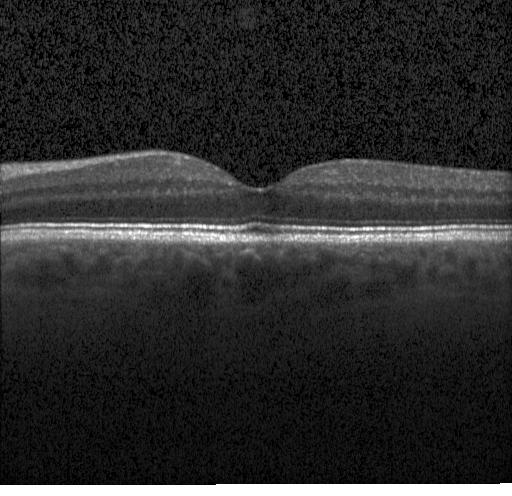

Spectral-domain OCT B-scan: no evidence of CNV, DME, or drusen.